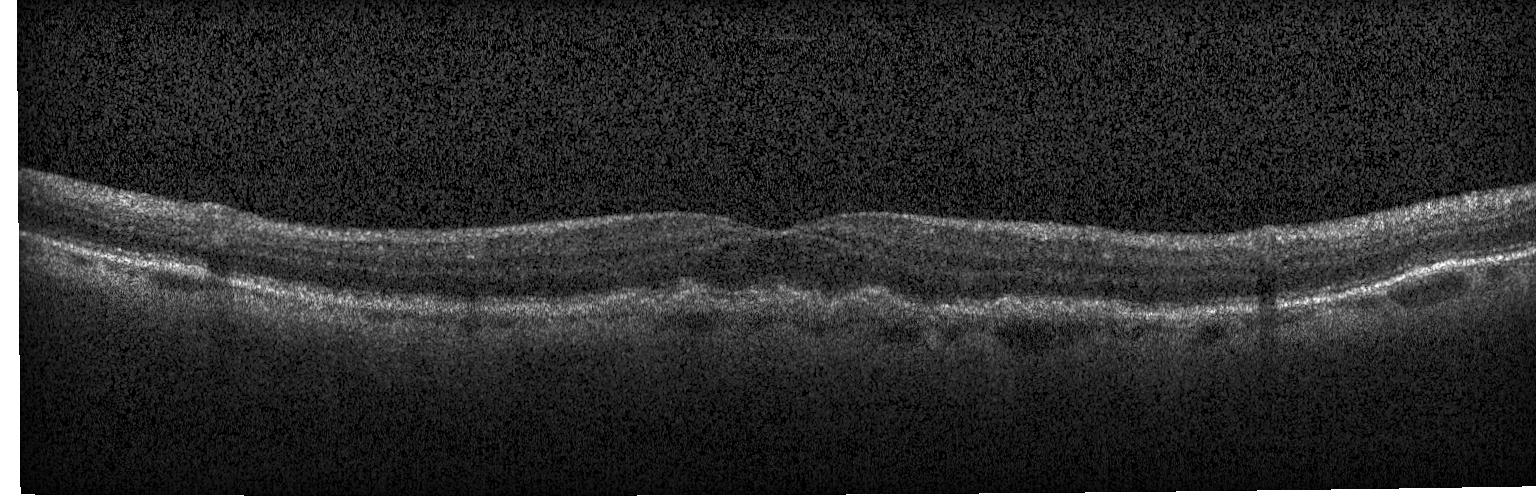

Macular OCT: choroidal neovascularization.